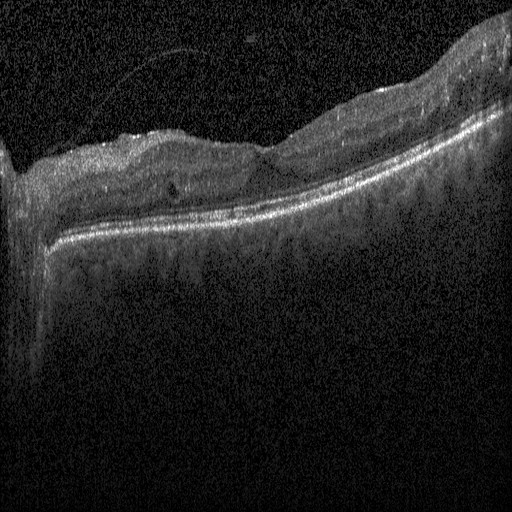 OCT B-scan showing diabetic macular edema.